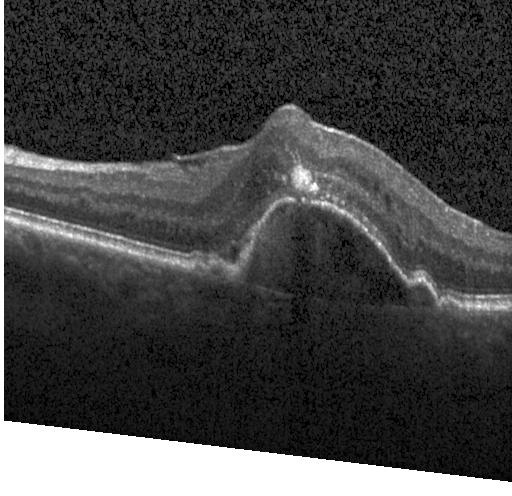
Optical coherence tomography B-scan, spectral-domain OCT, centered on the fovea, Heidelberg Spectralis.
The scan shows CNV.